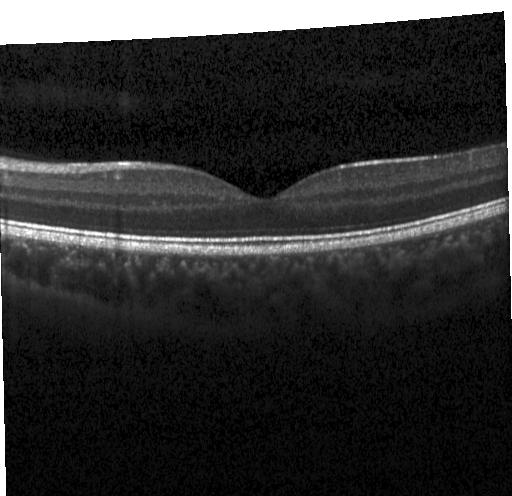
SD-OCT, horizontal scan through the fovea, OCT line scan — This B-scan demonstrates no choroidal neovascularization, diabetic macular edema, or drusen.